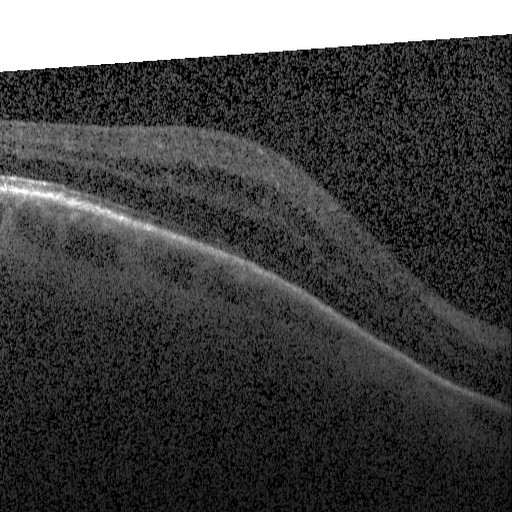
Diagnosis: DME.